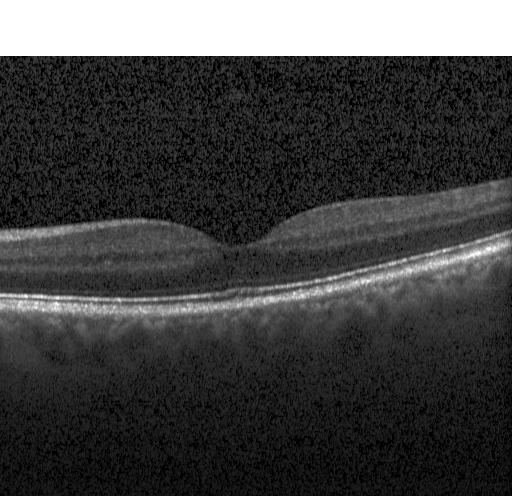 Instrument: Heidelberg Spectralis · horizontal scan through the fovea · OCT line scan. Finding: no evidence of choroidal neovascularization, diabetic macular edema, or drusen.